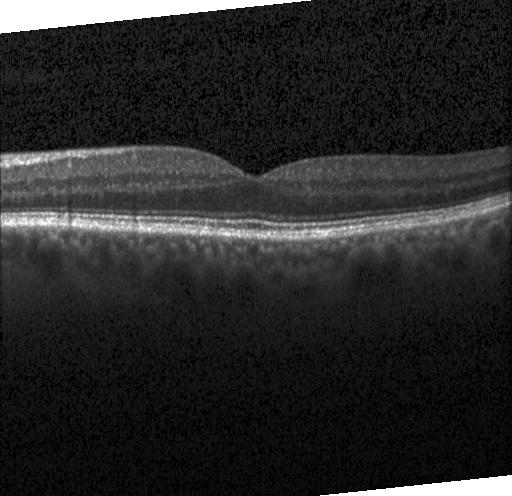 Heidelberg Spectralis · SD-OCT · OCT line scan · through the macula — Neither CNV, DME, nor drusen.